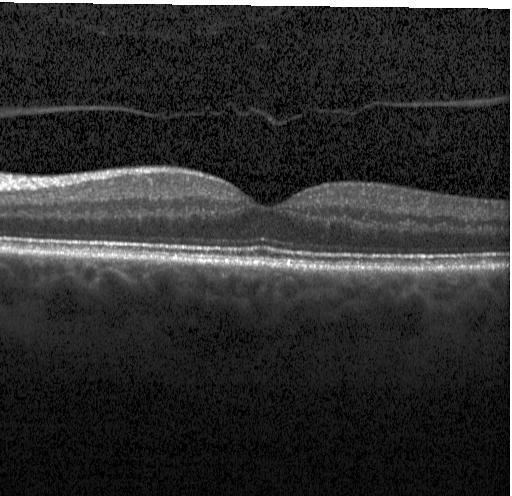
OCT line scan
Finding: no evidence of choroidal neovascularization, diabetic macular edema, or drusen.